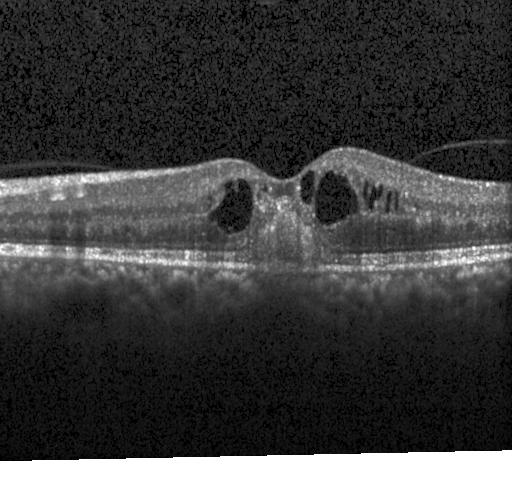

Retinal OCT B-scan.
Diagnosis: a choroidal neovascular membrane.